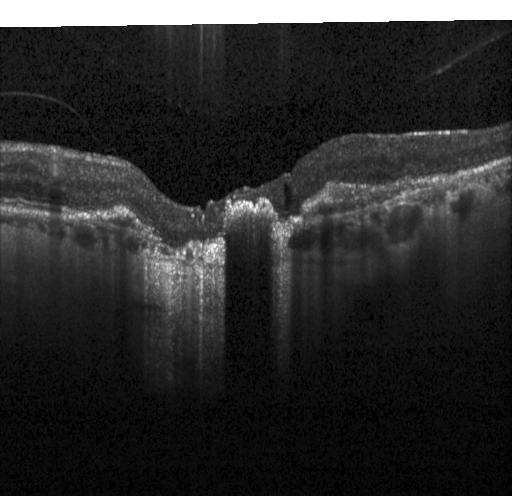
OCT B-scan — Macular OCT: a choroidal neovascular membrane.